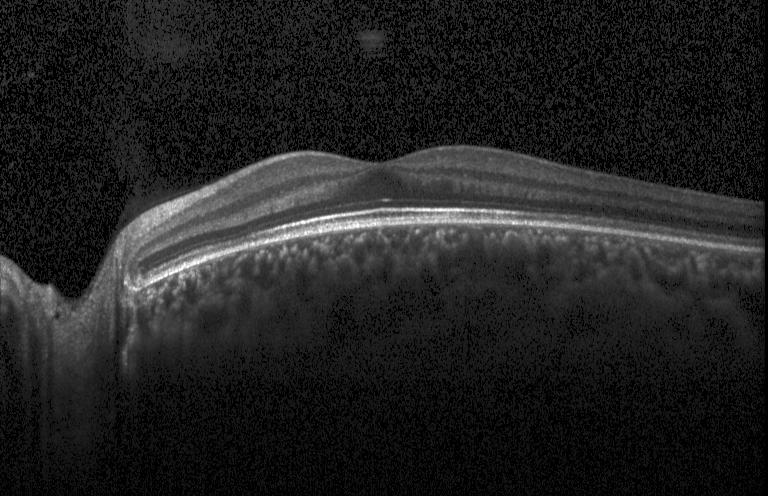 Retinal OCT cross-section.
This B-scan demonstrates no choroidal neovascularization, diabetic macular edema, or drusen.